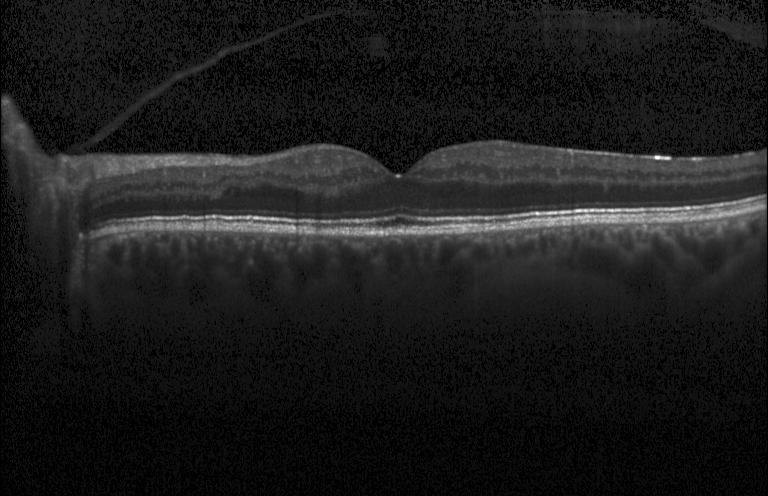

OCT line scan; through the macula; SD-OCT. Finding: neither CNV, DME, nor drusen.